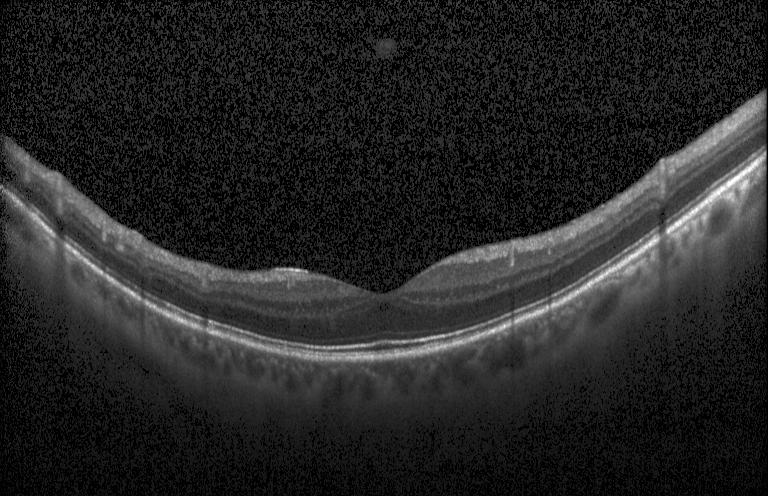

Horizontal scan through the fovea. OCT B-scan. Instrument: Heidelberg Spectralis. Spectral-domain optical coherence tomography. No evidence of choroidal neovascularization, diabetic macular edema, or drusen.